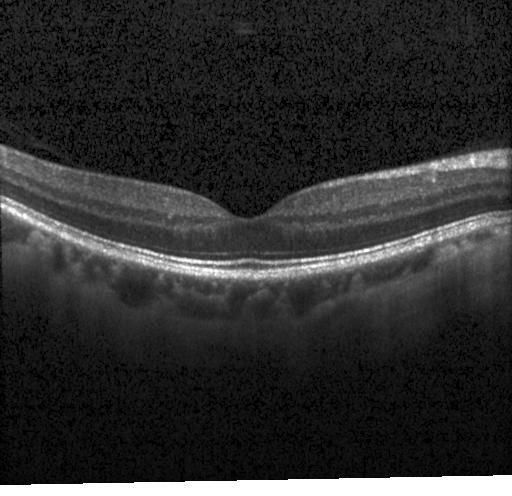
Optical coherence tomography B-scan, macular scan, acquired on a Heidelberg Spectralis — Macular OCT: no evidence of choroidal neovascularization, diabetic macular edema, or drusen.